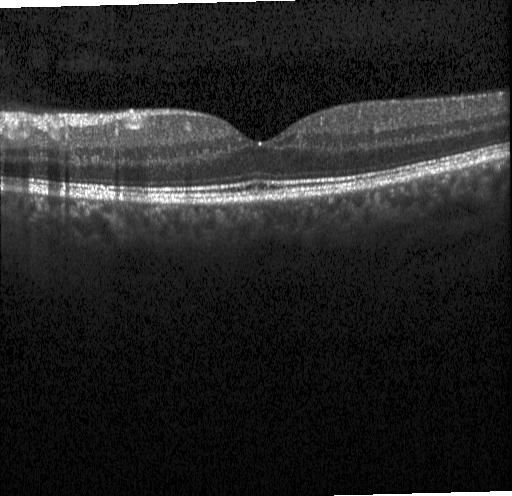

Retinal OCT cross-section. Macular scan. Instrument: Heidelberg Spectralis.
This B-scan demonstrates no evidence of choroidal neovascularization, diabetic macular edema, or drusen.